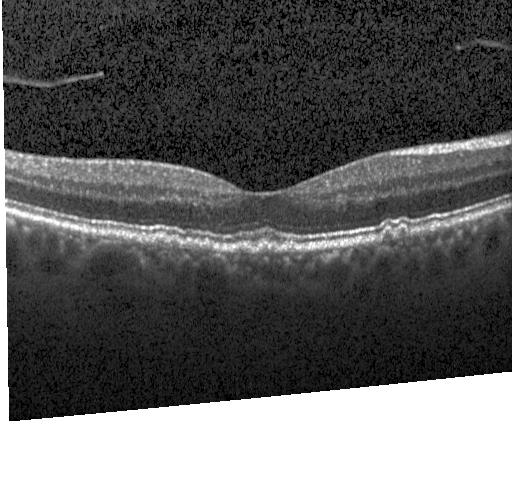

Assessment: multiple drusen.